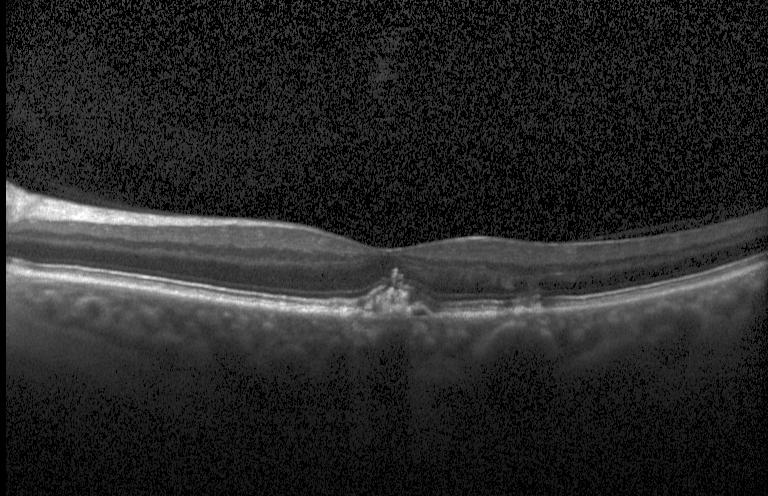 Retinal OCT cross-section, spectral-domain OCT, instrument: Heidelberg Spectralis, horizontal scan through the fovea — Assessment: a choroidal neovascular membrane.